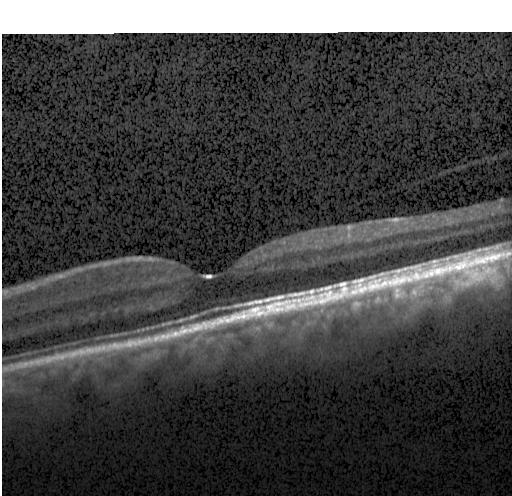
Optical coherence tomography scan
Finding: no CNV, no DME, and no drusen.